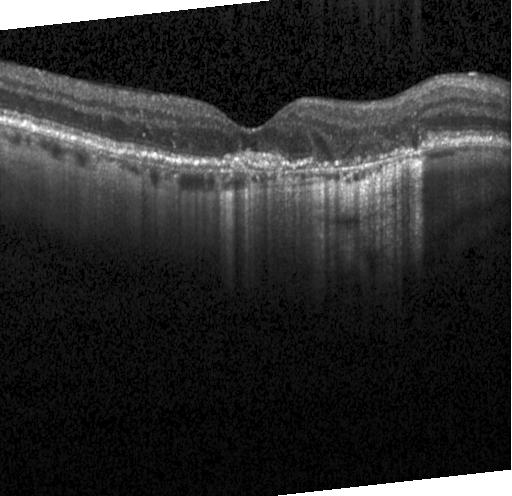 Through the macula · retinal OCT B-scan.
Diagnosis: choroidal neovascularization (CNV).